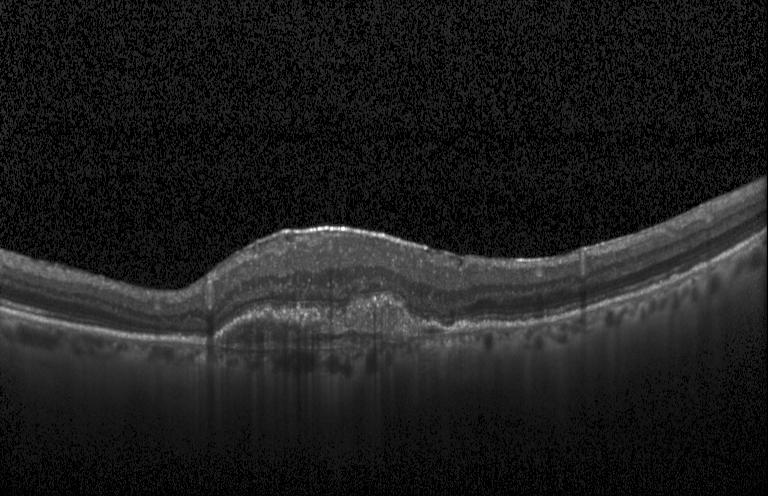 Instrument: Heidelberg Spectralis, spectral-domain OCT, optical coherence tomography B-scan, horizontal scan through the fovea.
This B-scan demonstrates a choroidal neovascular membrane.